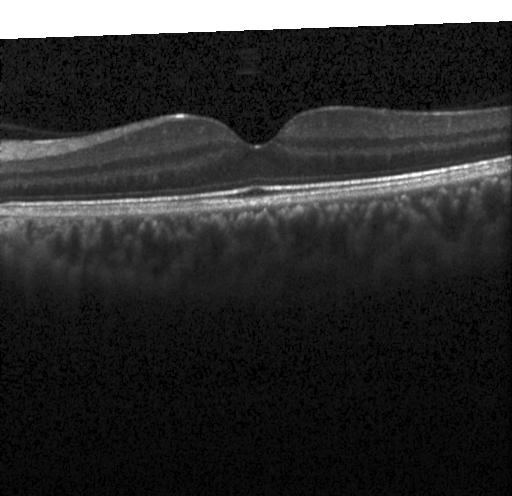

Acquired on a Heidelberg Spectralis; optical coherence tomography scan; SD-OCT
Diagnosis: no choroidal neovascularization, diabetic macular edema, or drusen.